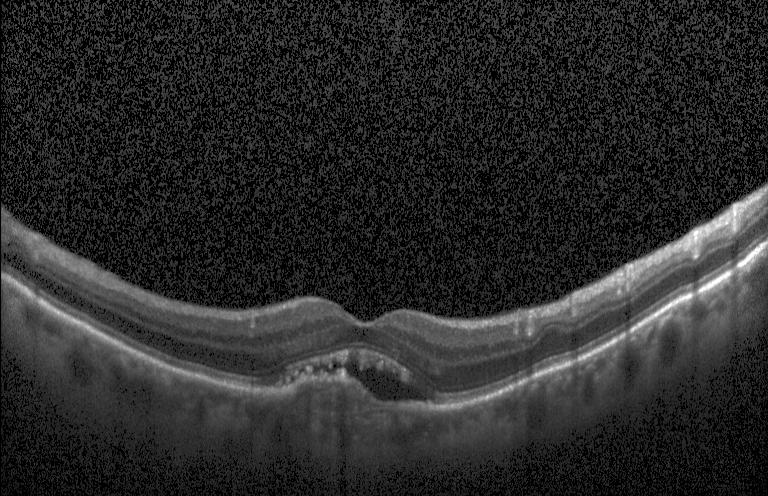
Finding: choroidal neovascularization (CNV).